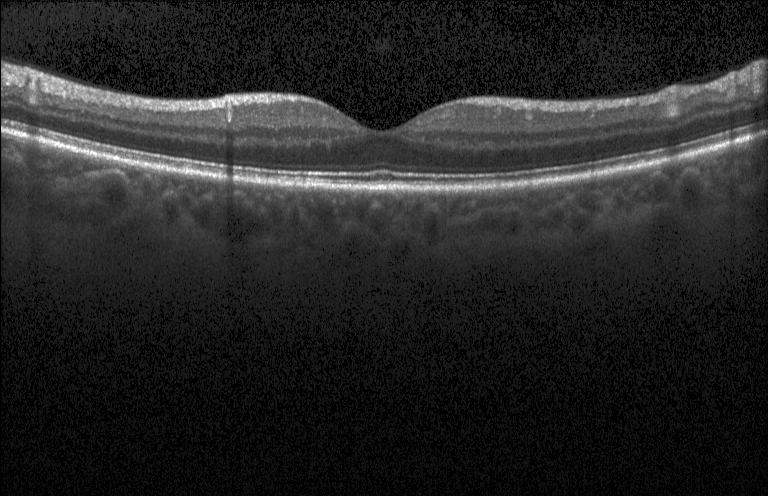

The scan shows no choroidal neovascularization, diabetic macular edema, or drusen.